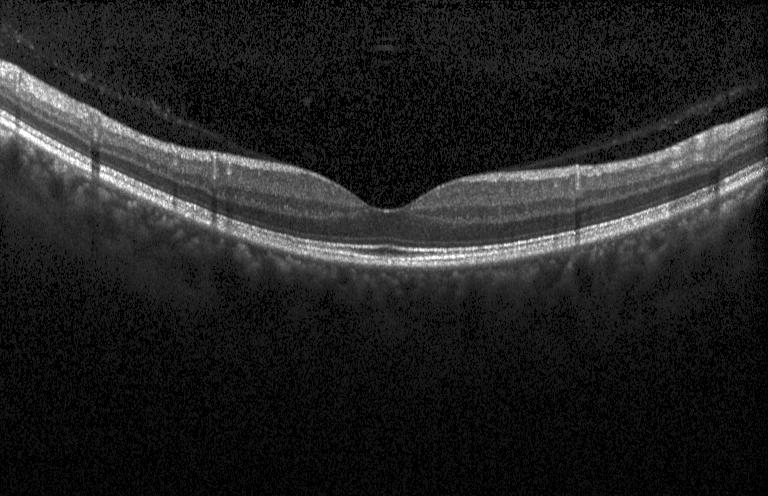

OCT line scan; Heidelberg Spectralis OCT system; through the macula
Diagnosis: no CNV, DME, or drusen.